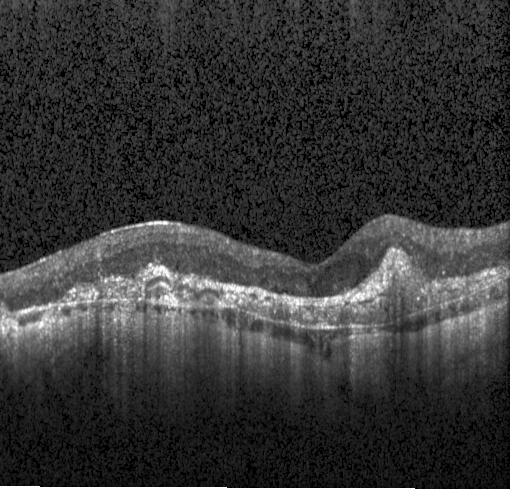
OCT line scan; Heidelberg Spectralis; SD-OCT.
Finding: a choroidal neovascular membrane.